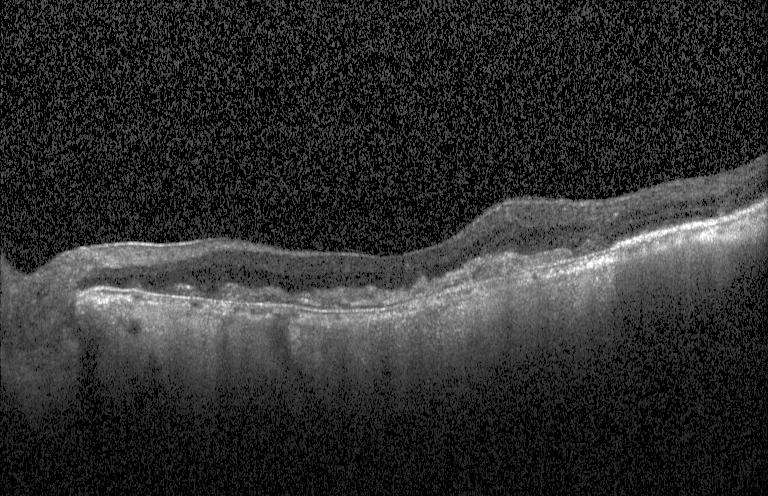 Optical coherence tomography scan; centered on the fovea.
Dx: a choroidal neovascular membrane.